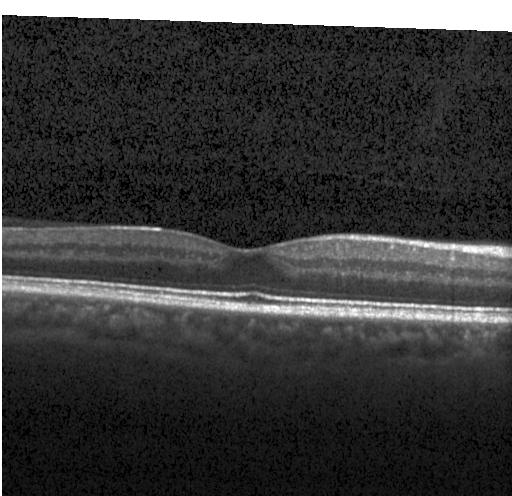
Retinal OCT cross-section showing no CNV, DME, or drusen.